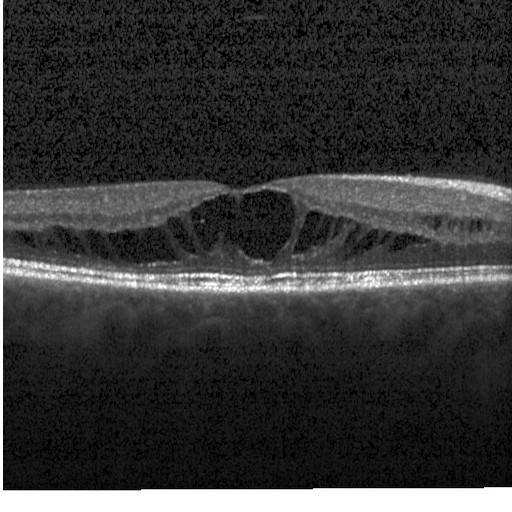 OCT finding: diabetic macular edema (DME).